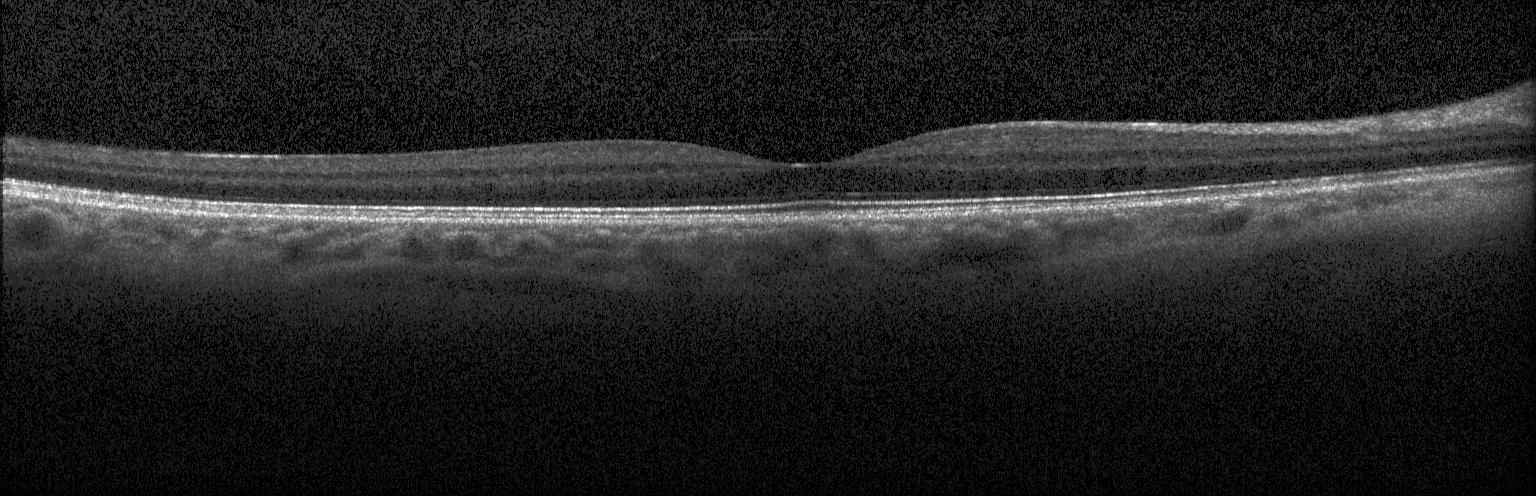
Finding: no evidence of CNV, DME, or drusen.